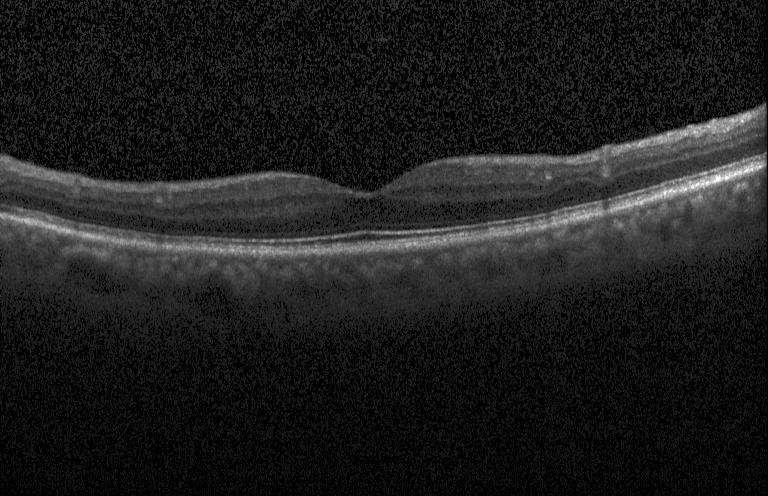 Optical coherence tomography scan.
No evidence of CNV, DME, or drusen.